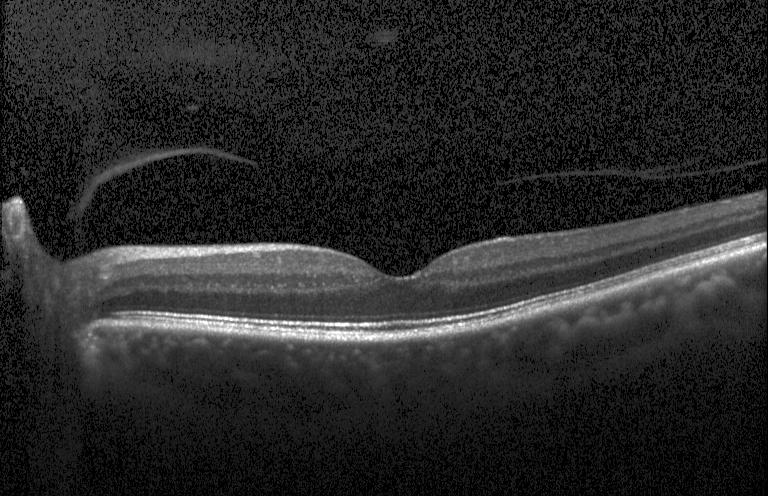

Optical coherence tomography scan; spectral-domain OCT. Diagnosis: no CNV, DME, or drusen.